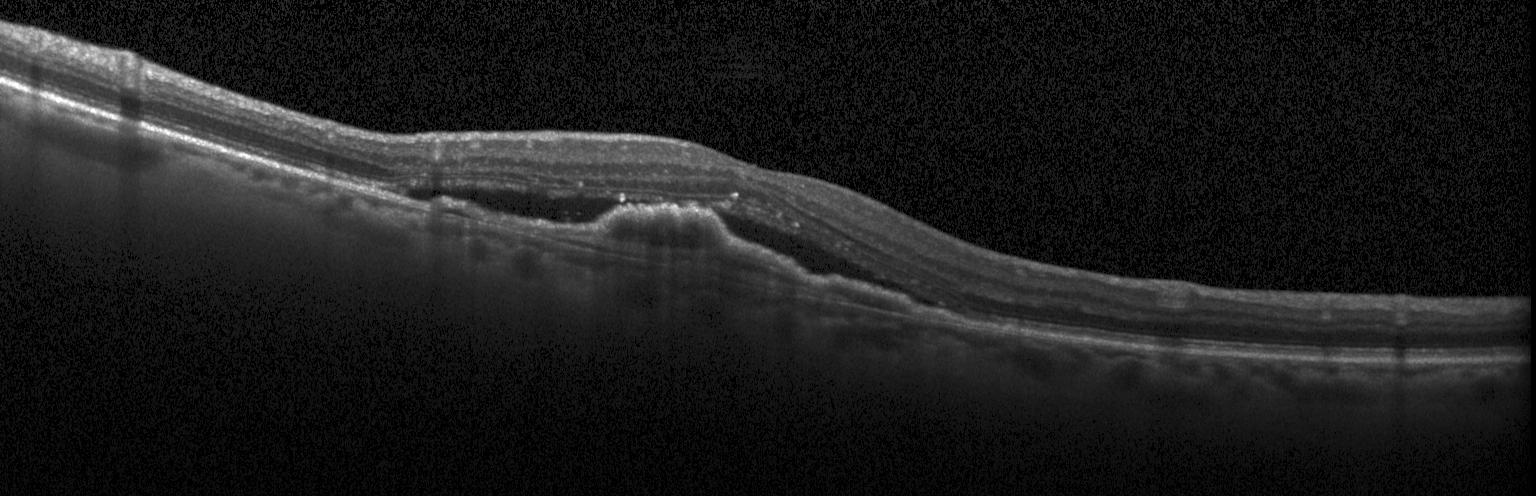
The scan shows CNV.